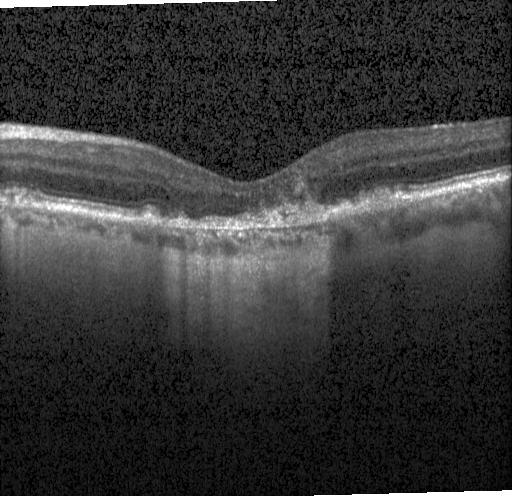 Optical coherence tomography scan · fovea-centered · Heidelberg Spectralis — Macular OCT: CNV.